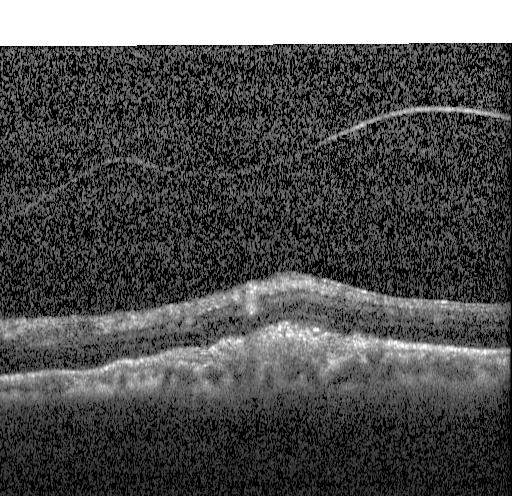
Retinal OCT cross-section
Diagnosis: a choroidal neovascular membrane.